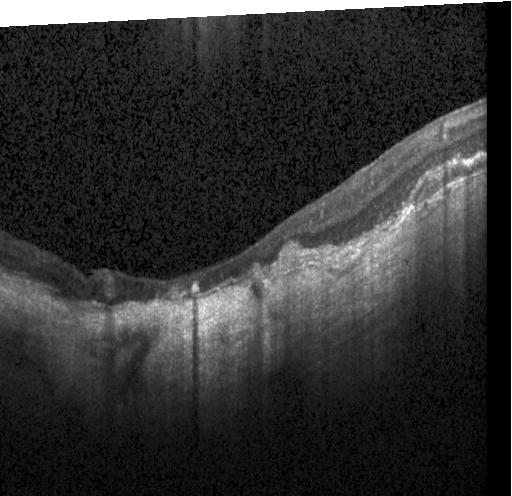
Centered on the fovea · OCT B-scan.
Impression: a choroidal neovascular membrane.